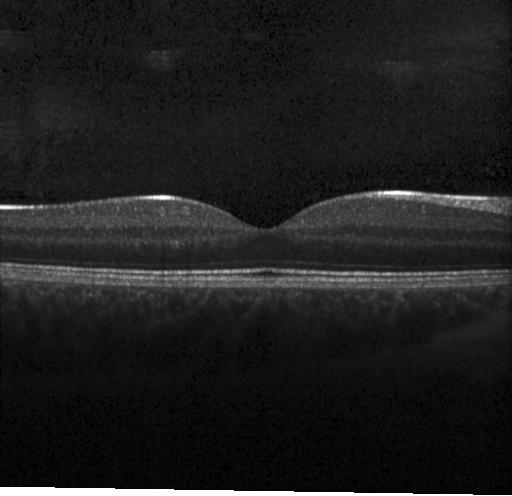

Spectral-domain optical coherence tomography · centered on the fovea · retinal OCT B-scan.
OCT finding: no evidence of choroidal neovascularization, diabetic macular edema, or drusen.